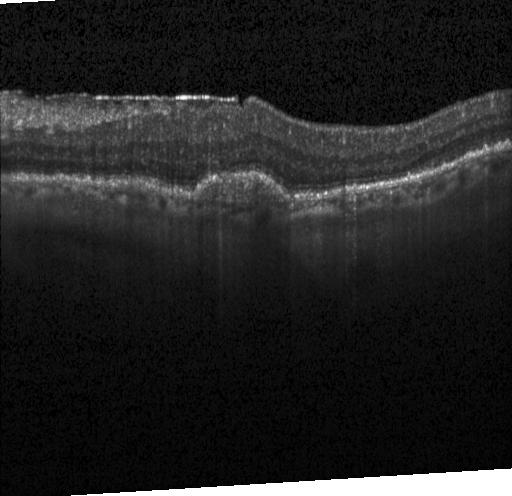
Optical coherence tomography scan
Impression: choroidal neovascularization (CNV).